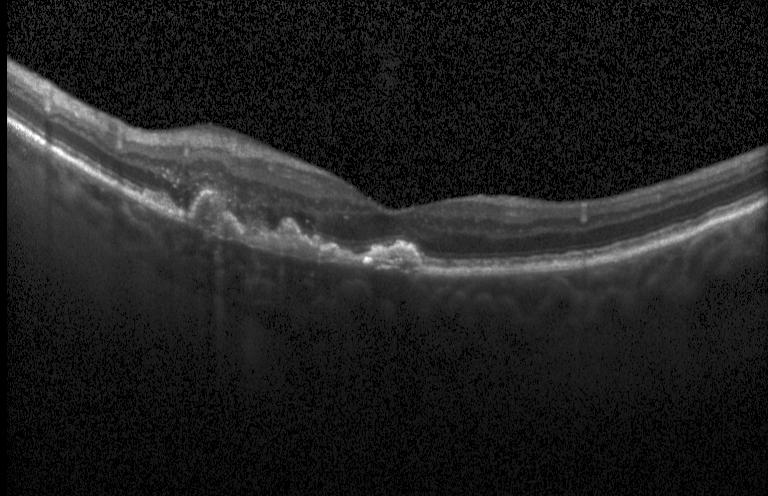 Retinal OCT cross-section, spectral-domain OCT.
Dx: a choroidal neovascular membrane.